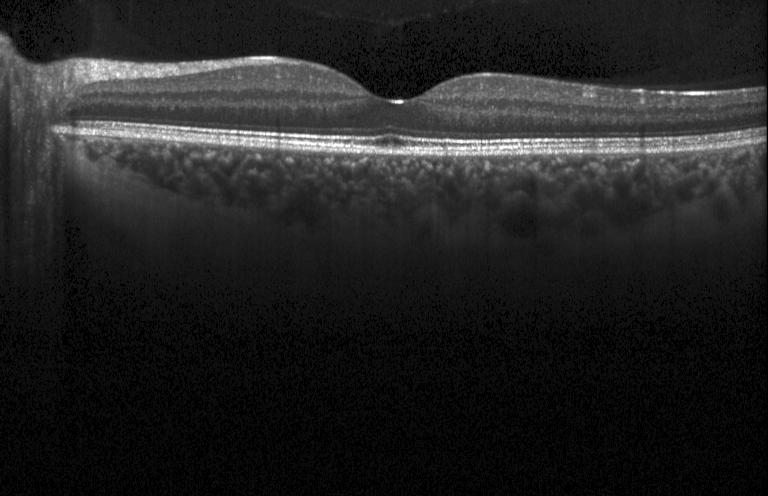
SD-OCT. OCT B-scan. Diagnosis: no evidence of choroidal neovascularization, diabetic macular edema, or drusen.